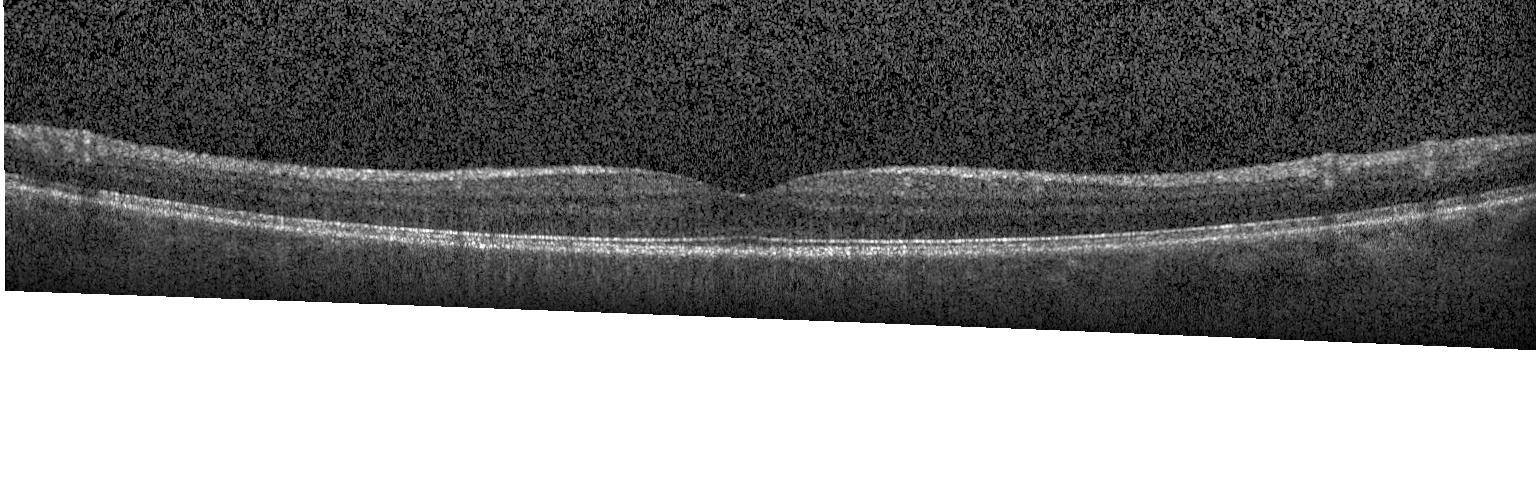

OCT finding: no evidence of choroidal neovascularization, diabetic macular edema, or drusen.